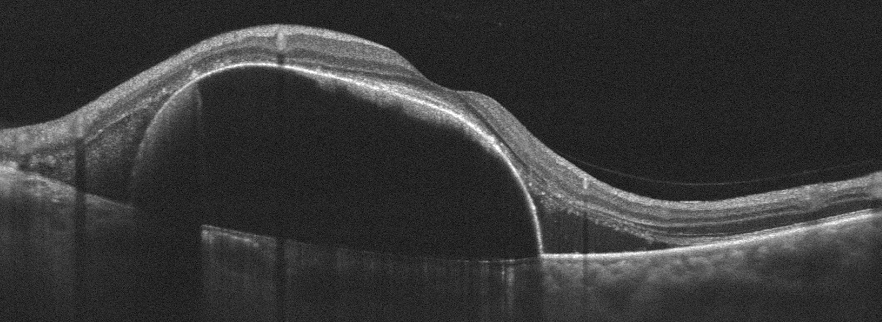
OCT line scan; OD
Macular OCT: age-related macular degeneration (AMD).